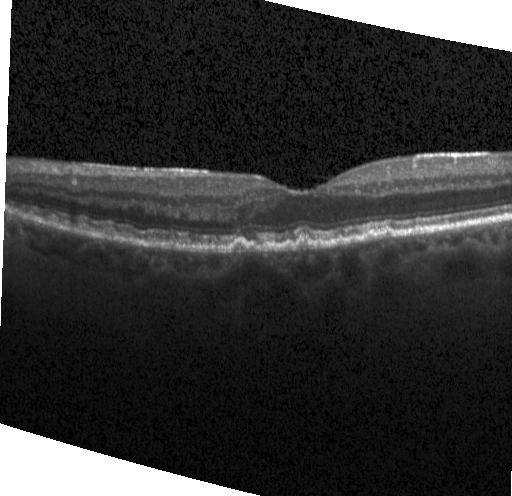
Impression: multiple drusen.